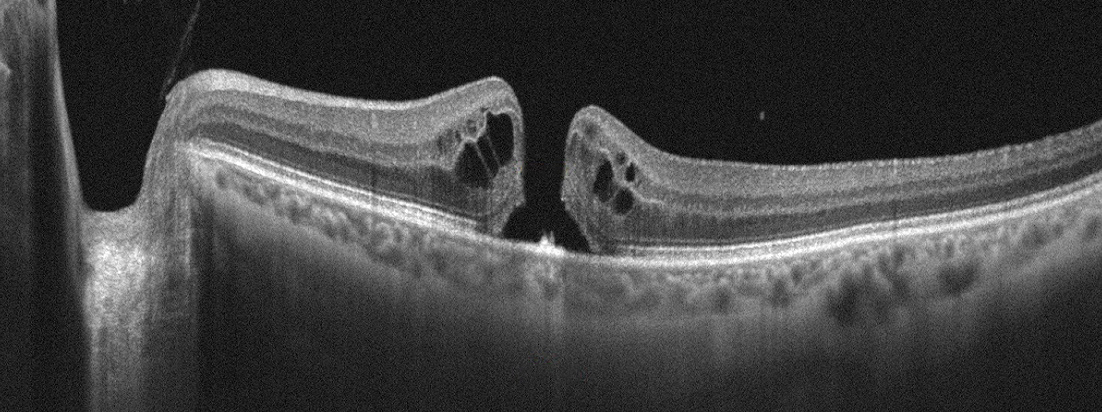 Retinal OCT cross-section. Impression: vitreomacular interface disease.